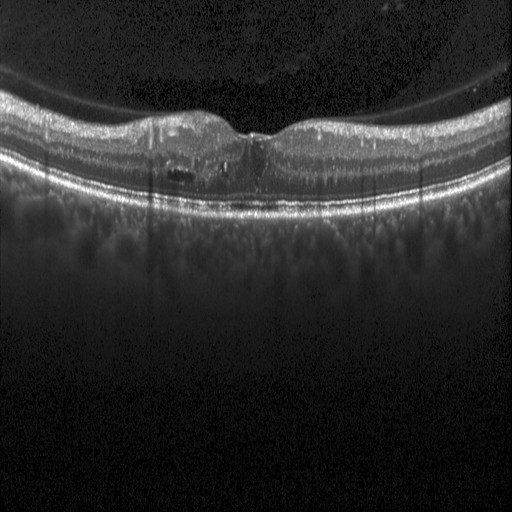

Retinal OCT cross-section showing DME.